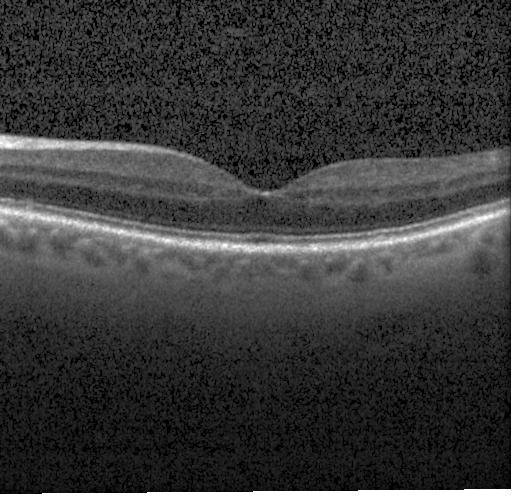
Through the macula; Heidelberg Spectralis OCT system; optical coherence tomography scan.
The scan shows no choroidal neovascularization, diabetic macular edema, or drusen.